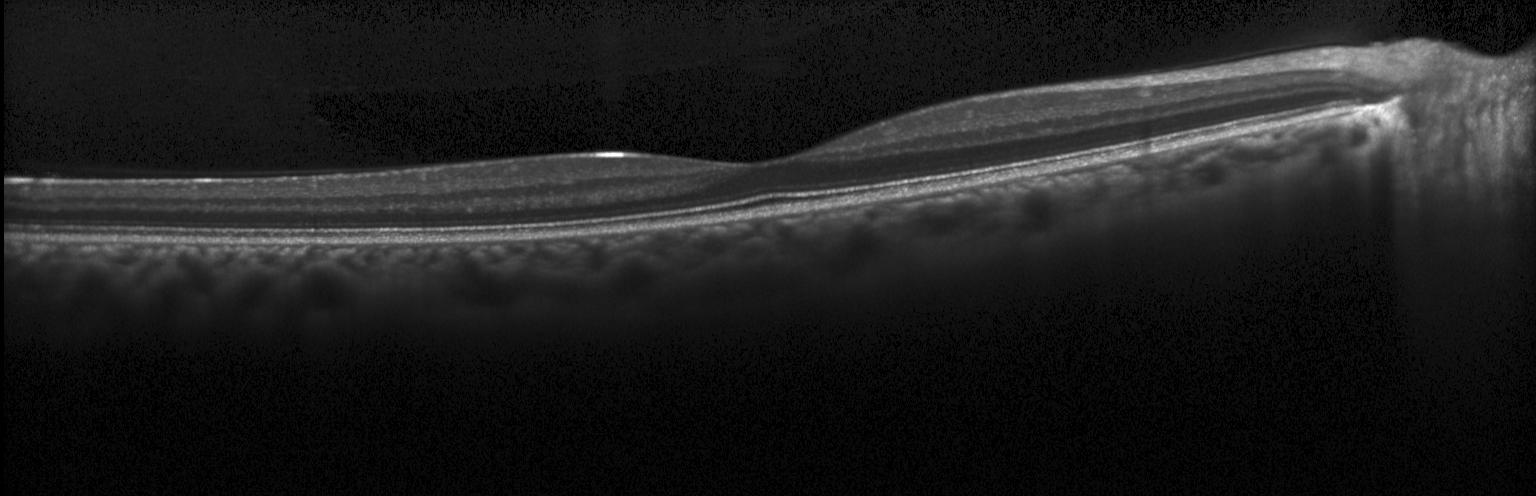 SD-OCT, retinal OCT B-scan — Macular OCT: neither choroidal neovascularization, diabetic macular edema, nor drusen.